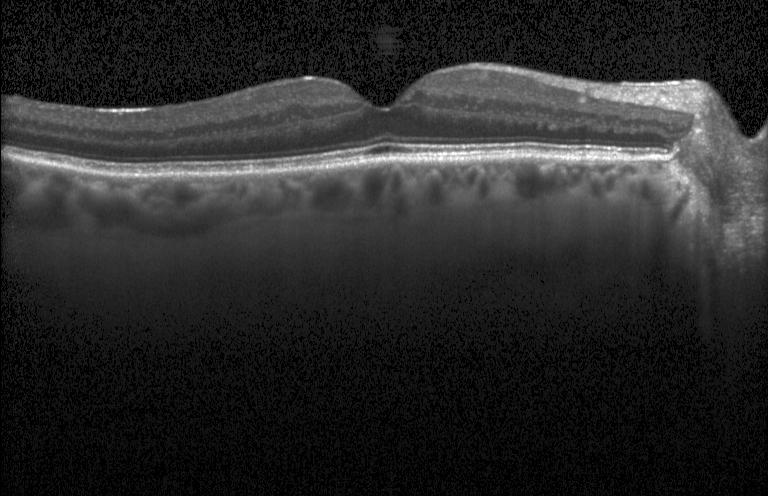

Horizontal scan through the fovea, SD-OCT, retinal OCT cross-section
Dx: no choroidal neovascularization, no diabetic macular edema, and no drusen.